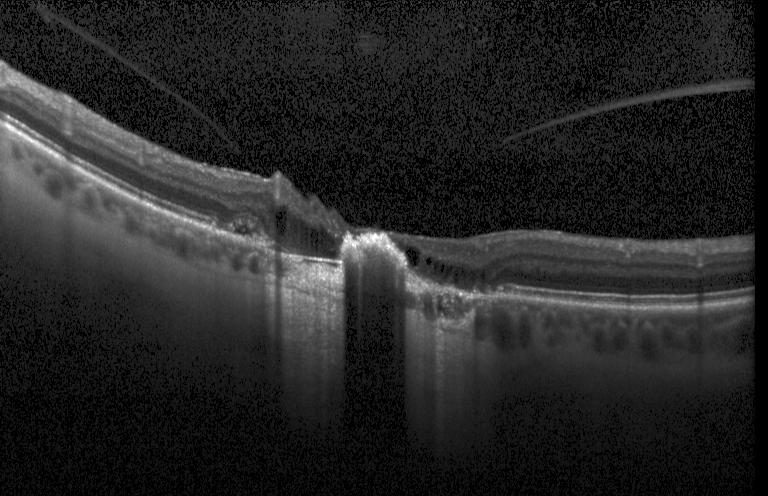 This B-scan demonstrates choroidal neovascularization.